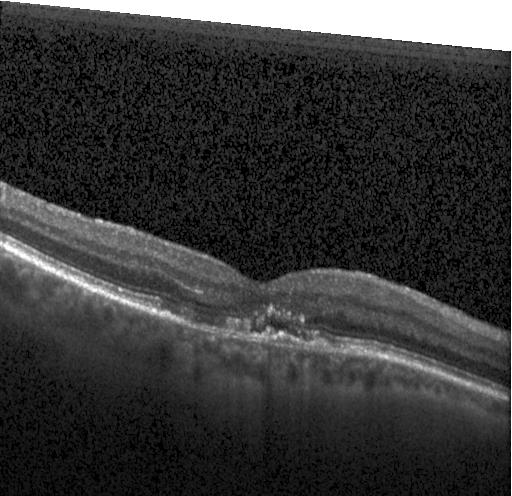
Macular OCT: choroidal neovascularization (CNV).